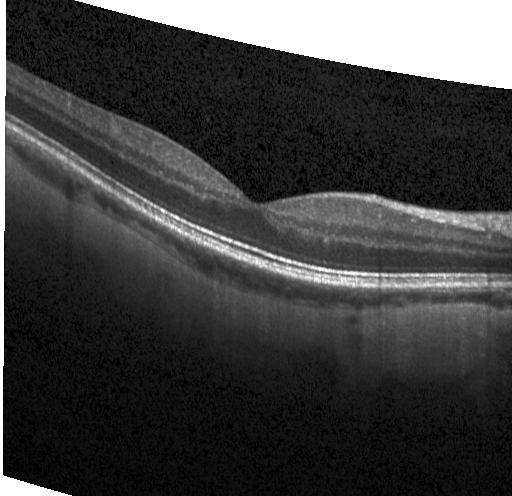
Macular scan. Spectral-domain OCT. OCT B-scan. Heidelberg Spectralis
No evidence of choroidal neovascularization, diabetic macular edema, or drusen.